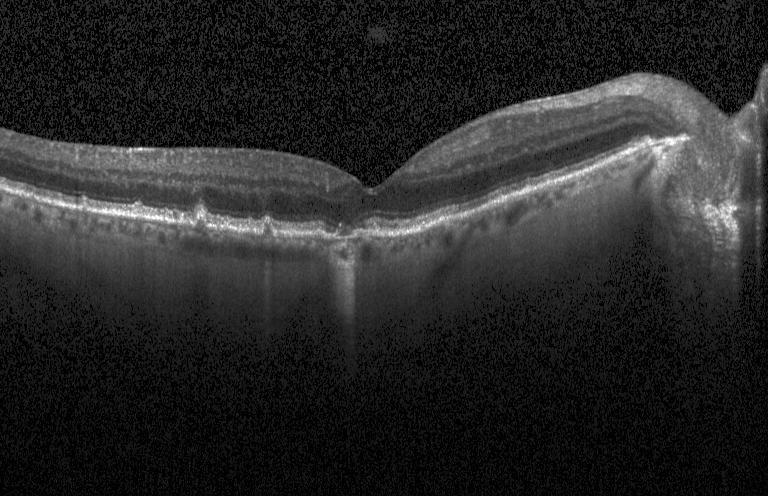 OCT line scan · fovea-centered · acquired on a Heidelberg Spectralis · spectral-domain OCT — Finding: drusen.